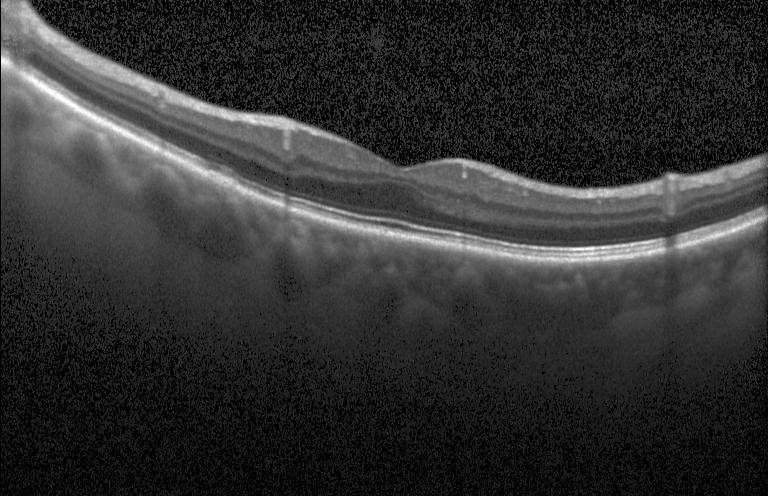 Spectral-domain OCT, optical coherence tomography B-scan.
No evidence of choroidal neovascularization, diabetic macular edema, or drusen.